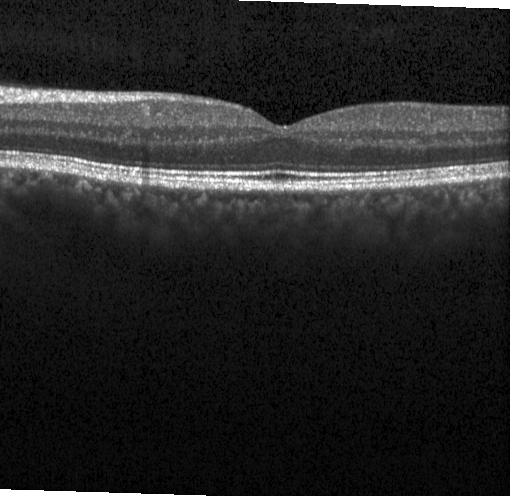
OCT line scan. Macular OCT: neither CNV, DME, nor drusen.